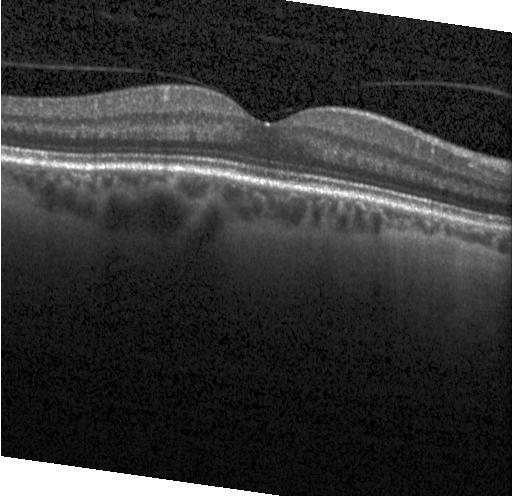 Retinal OCT cross-section
OCT finding: no choroidal neovascularization, no diabetic macular edema, and no drusen.